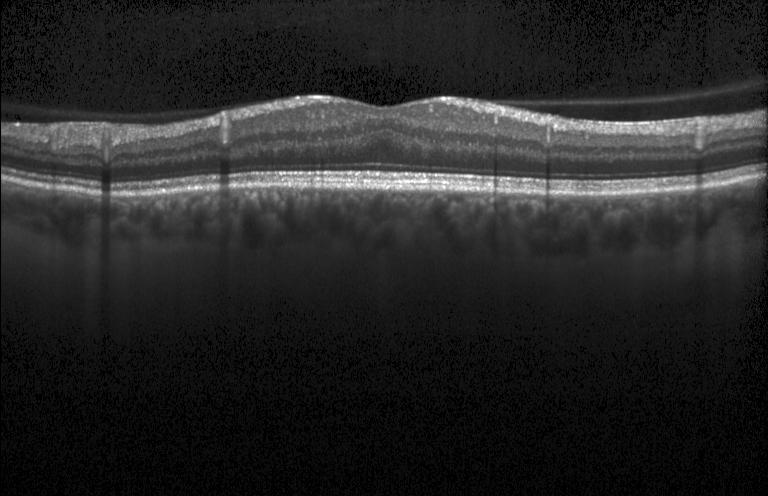
Impression: no choroidal neovascularization, diabetic macular edema, or drusen.